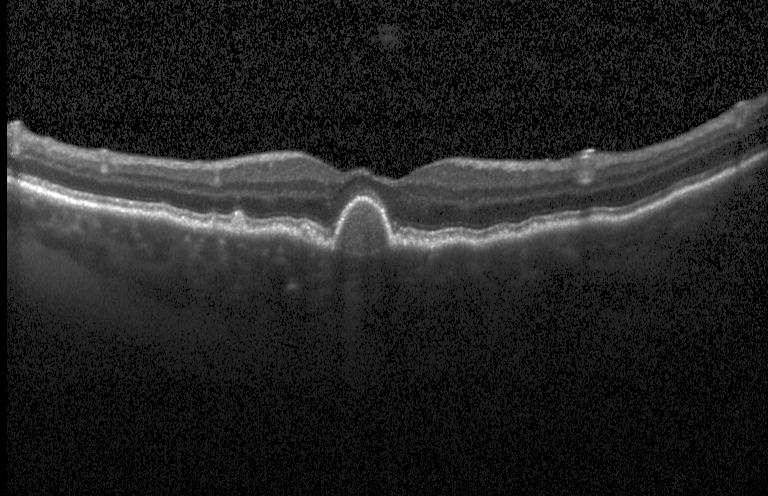 Retinal OCT B-scan, macular scan — Impression: drusen.